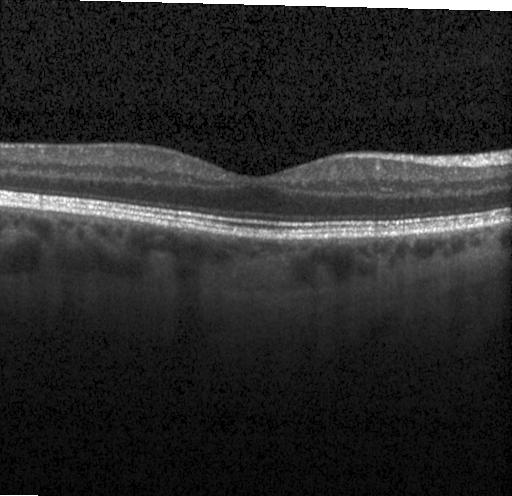
This B-scan demonstrates no evidence of choroidal neovascularization, diabetic macular edema, or drusen.